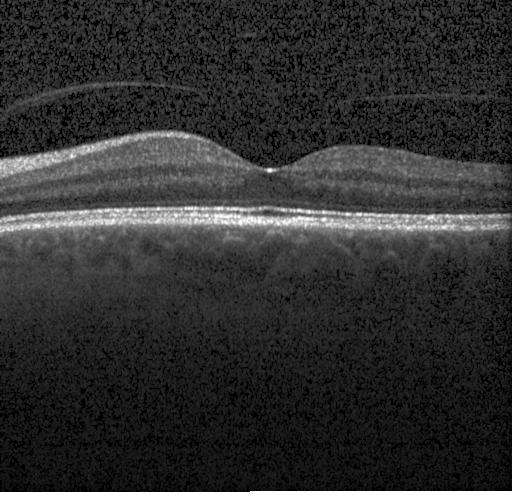 Heidelberg Spectralis OCT system, horizontal scan through the fovea, OCT line scan, spectral-domain OCT — OCT finding: no choroidal neovascularization, no diabetic macular edema, and no drusen.